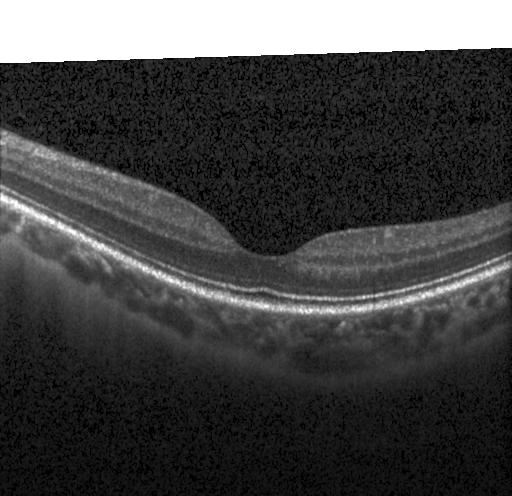 OCT B-scan
Assessment: no choroidal neovascularization, diabetic macular edema, or drusen.